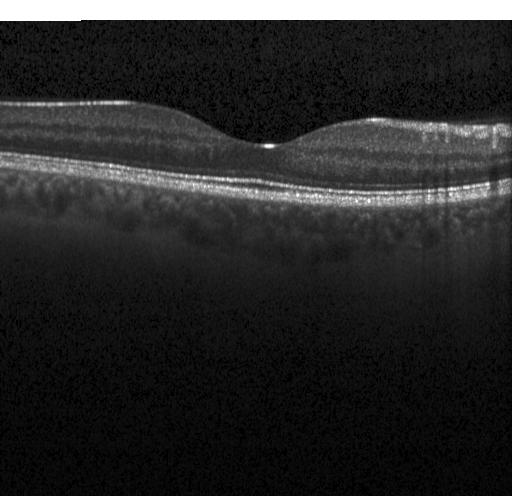 Fovea-centered; spectral-domain OCT; Heidelberg Spectralis OCT system; retinal OCT B-scan
Macular OCT: no evidence of choroidal neovascularization, diabetic macular edema, or drusen.